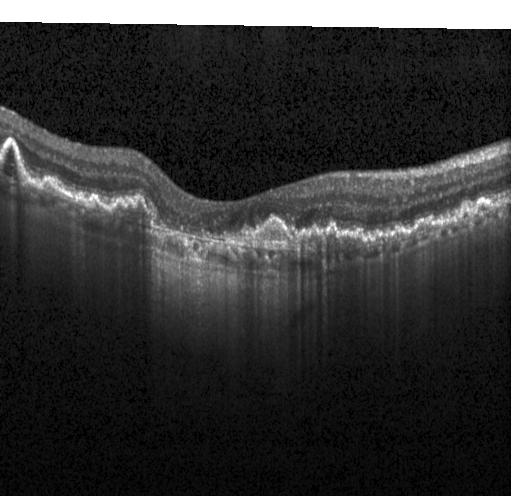

Spectral-domain optical coherence tomography, Heidelberg Spectralis OCT system, macular scan, optical coherence tomography scan
Finding: a choroidal neovascular membrane.